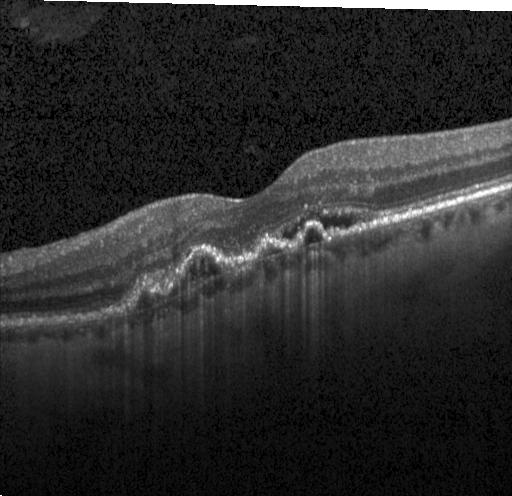

Diagnosis: a choroidal neovascular membrane.